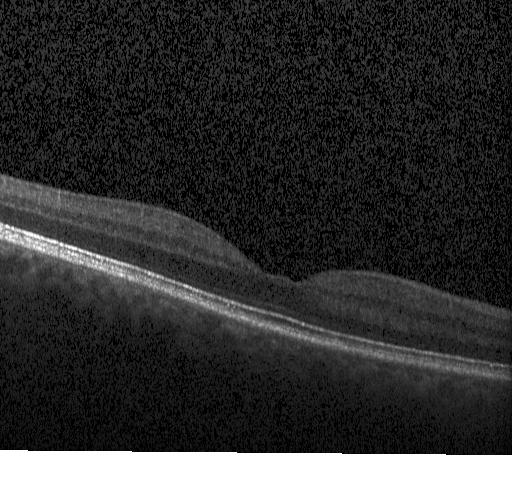

Acquired on a Heidelberg Spectralis · optical coherence tomography B-scan — No evidence of choroidal neovascularization, diabetic macular edema, or drusen.